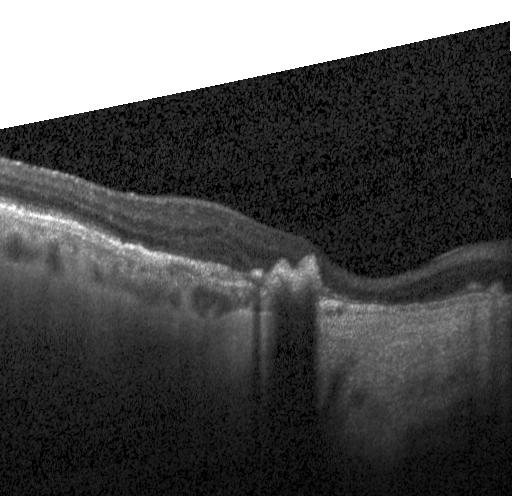 Dx: CNV.